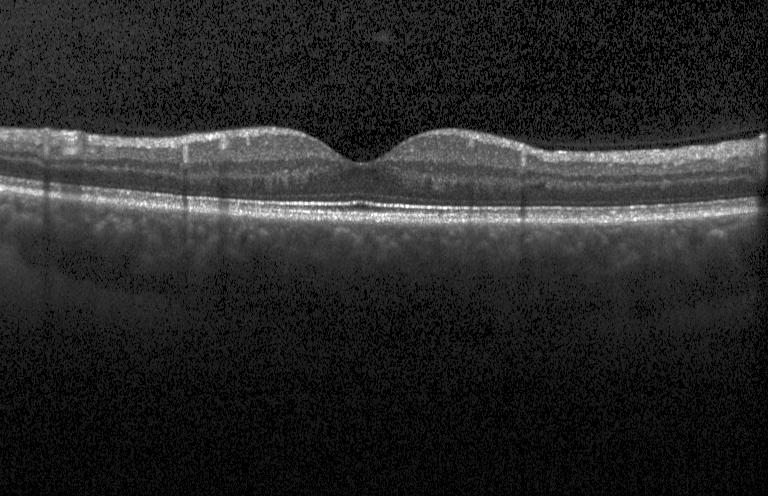
Centered on the fovea · OCT line scan — Diagnosis: no choroidal neovascularization, diabetic macular edema, or drusen.